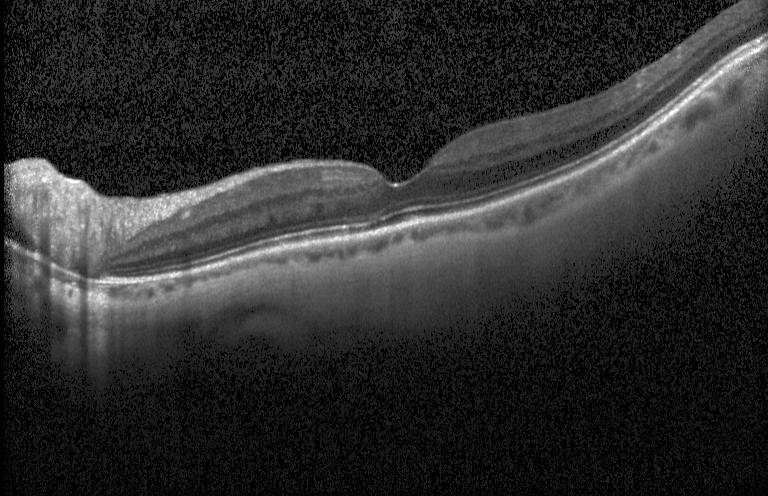

Impression: no evidence of choroidal neovascularization, diabetic macular edema, or drusen.